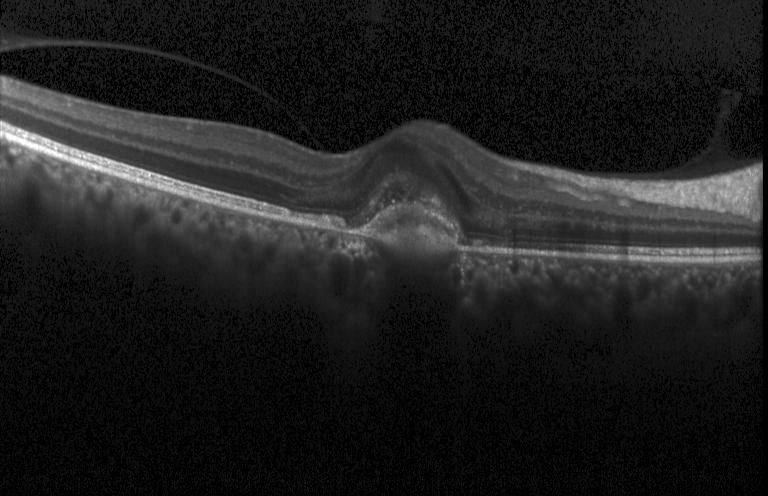 Optical coherence tomography B-scan · SD-OCT — The scan shows choroidal neovascularization (CNV).